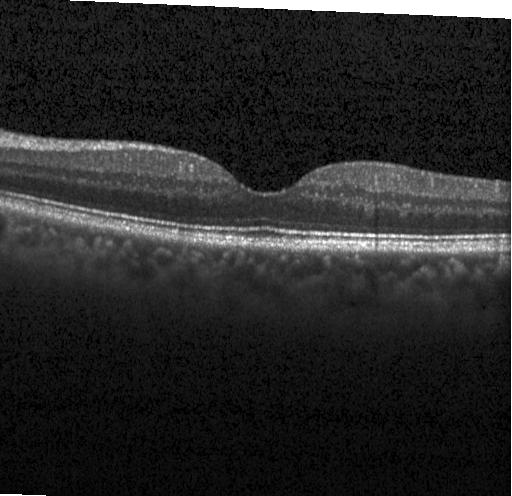

Macular scan · optical coherence tomography scan · SD-OCT · instrument: Heidelberg Spectralis
Finding: no evidence of choroidal neovascularization, diabetic macular edema, or drusen.